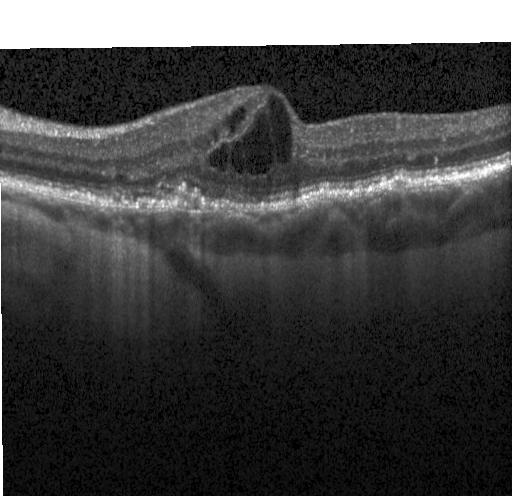 Macular OCT demonstrating choroidal neovascularization (CNV).